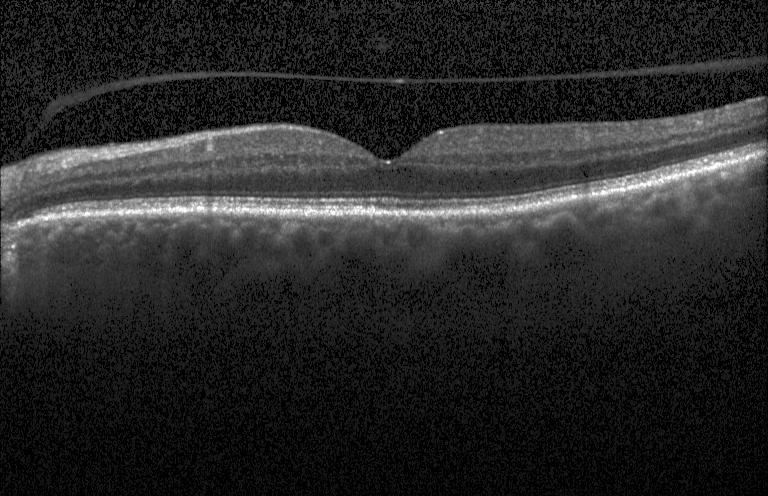
Spectral-domain OCT B-scan: no choroidal neovascularization, no diabetic macular edema, and no drusen.